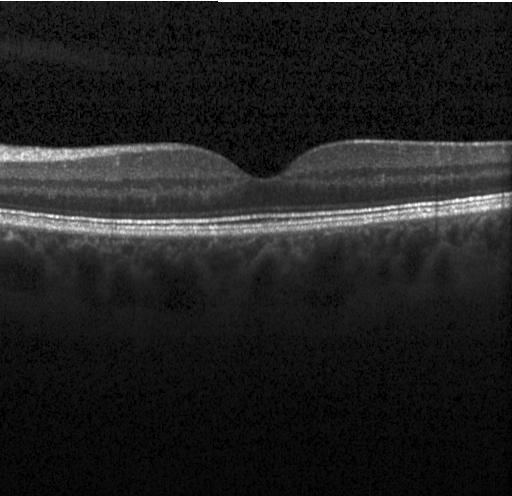 OCT B-scan. Through the macula.
Macular OCT: no evidence of choroidal neovascularization, diabetic macular edema, or drusen.